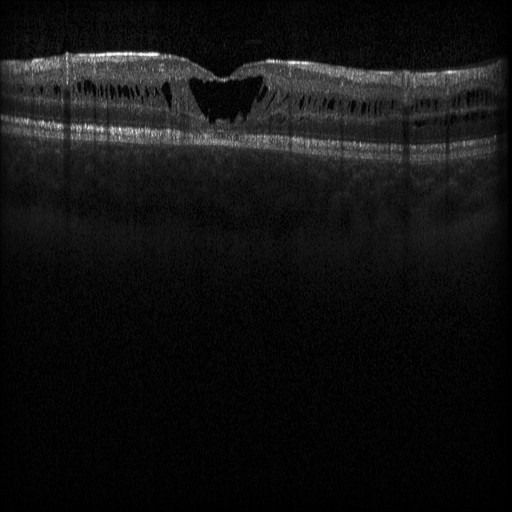

This B-scan demonstrates diabetic macular edema.